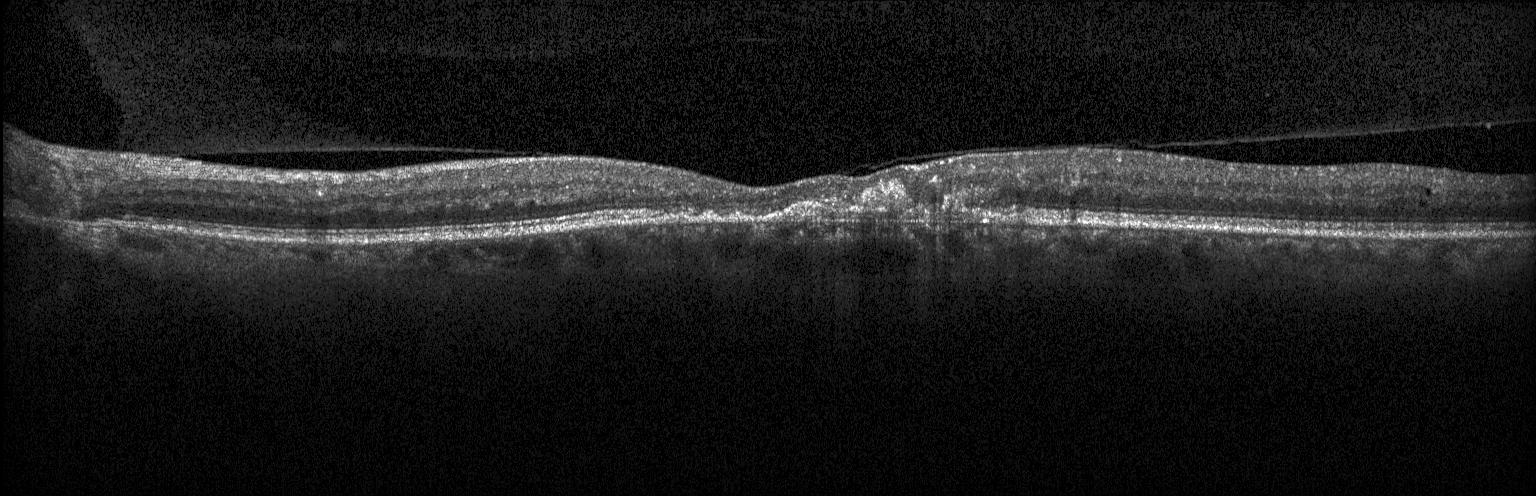

Optical coherence tomography scan · through the macula · Heidelberg Spectralis OCT system · SD-OCT.
Diagnosis: a choroidal neovascular membrane.